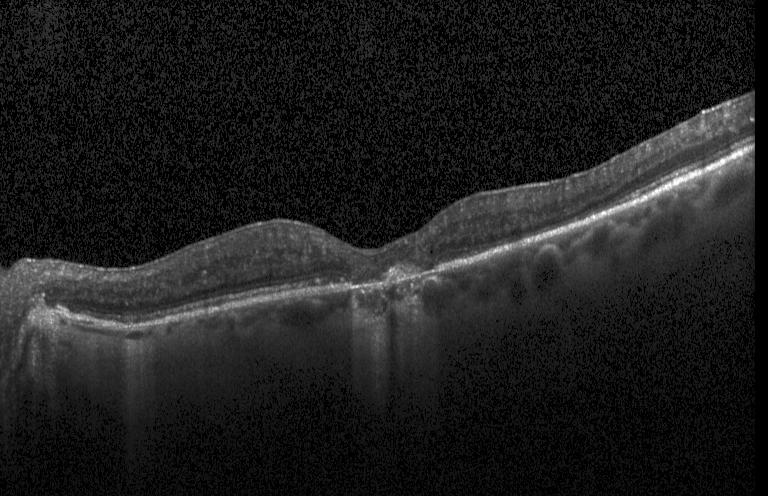 Diagnosis: a choroidal neovascular membrane.